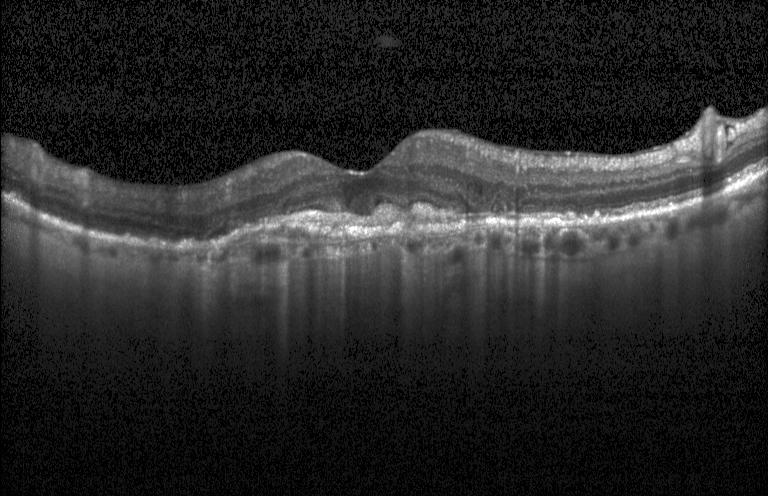

Diagnosis: a choroidal neovascular membrane.